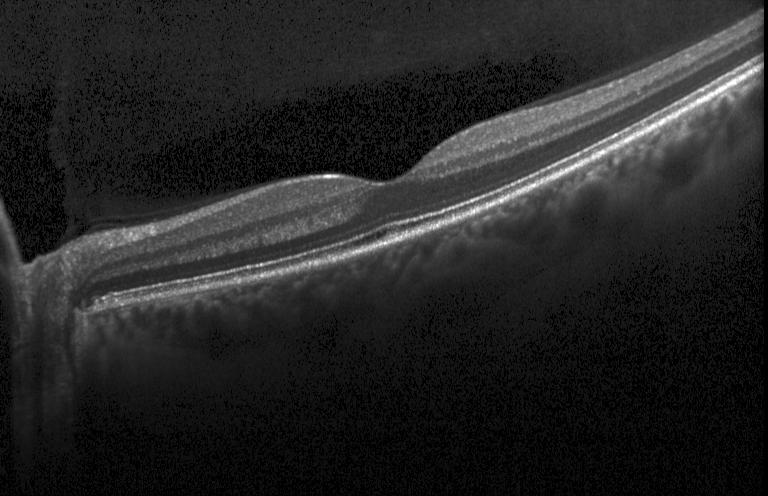
Finding: no choroidal neovascularization, diabetic macular edema, or drusen.